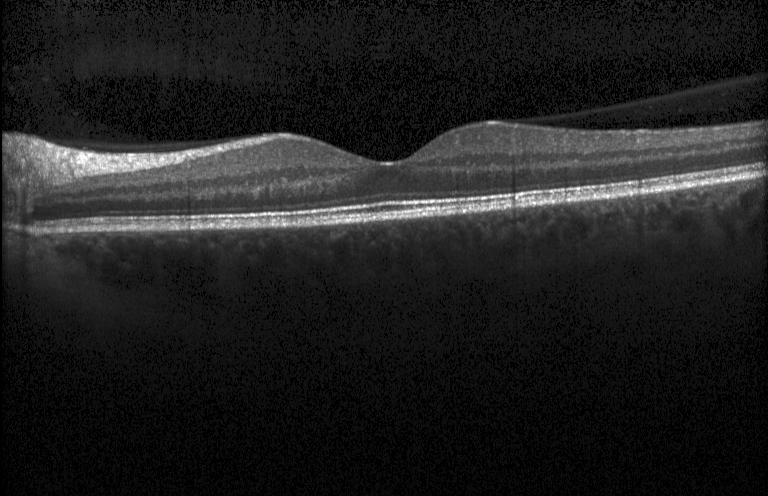
OCT B-scan showing neither choroidal neovascularization, diabetic macular edema, nor drusen.